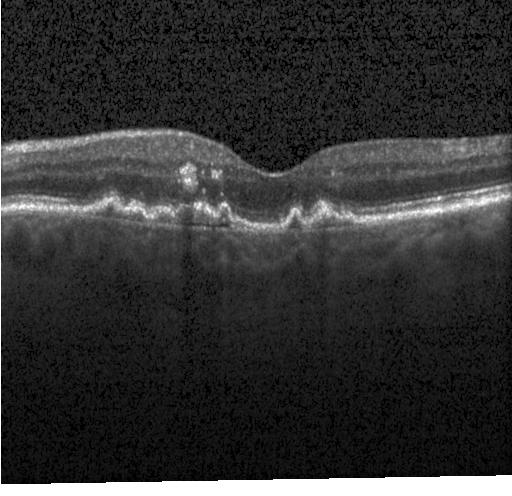

Macular scan. Acquired on a Heidelberg Spectralis. Optical coherence tomography scan. SD-OCT. Assessment: choroidal neovascularization (CNV).